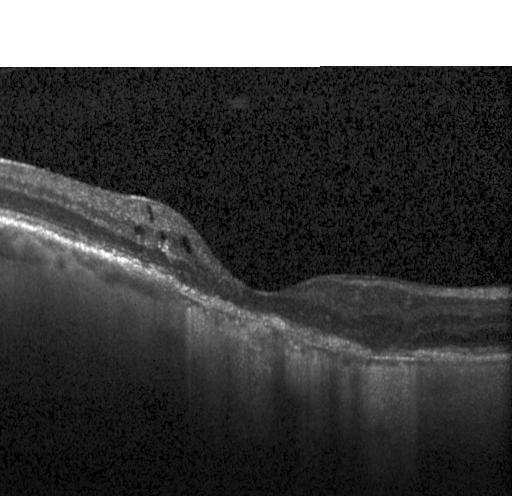
OCT B-scan, Heidelberg Spectralis OCT system
Dx: a choroidal neovascular membrane.